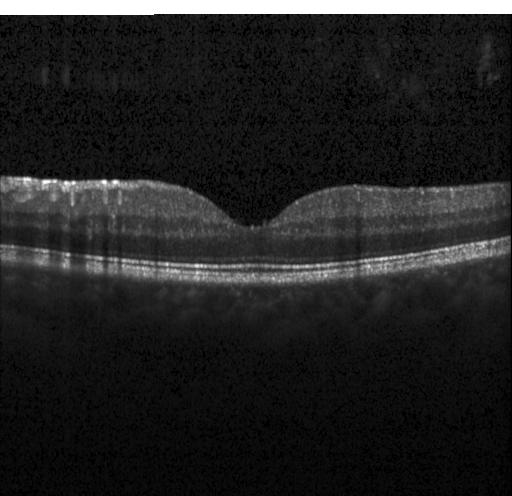
Retinal OCT cross-section; acquired on a Heidelberg Spectralis.
No choroidal neovascularization, no diabetic macular edema, and no drusen.